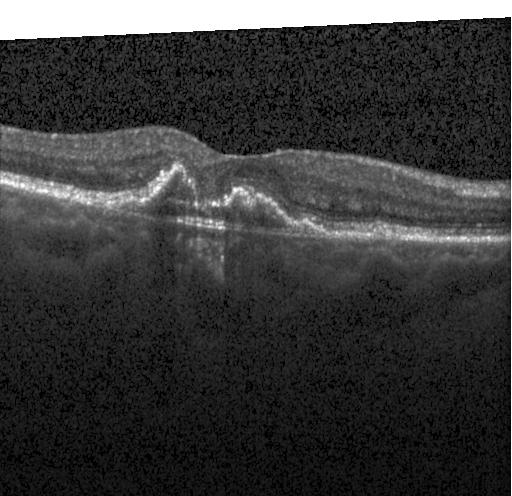
Finding: CNV.